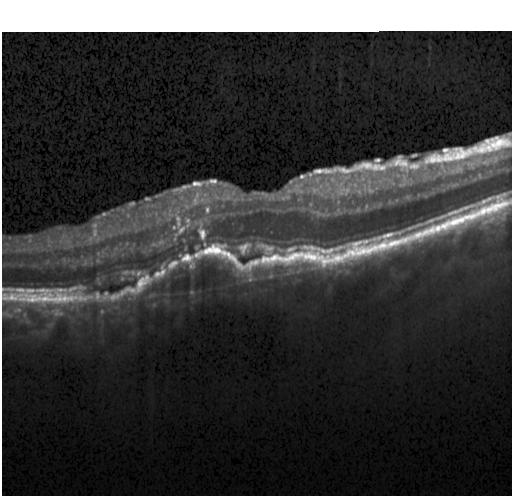 Diagnosis: choroidal neovascularization.